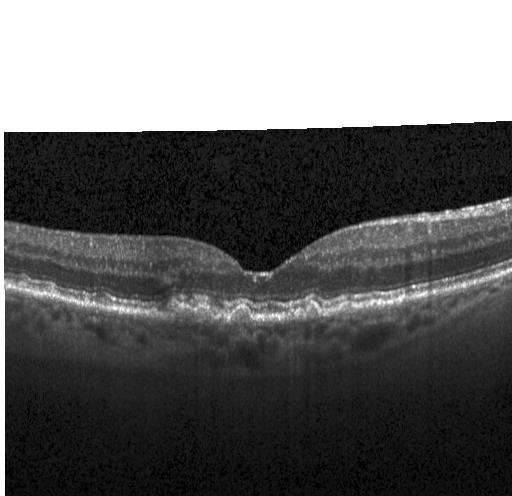 Diagnosis: drusen.